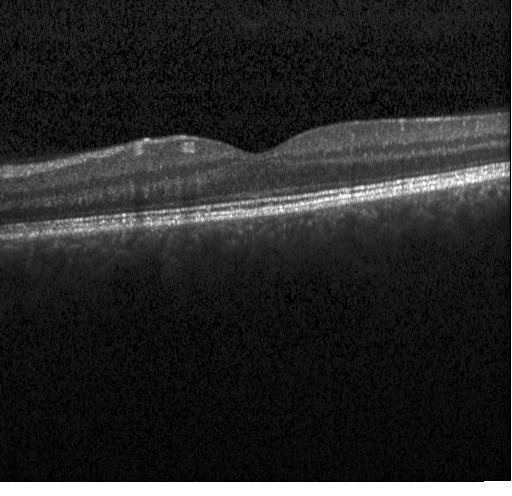 Retinal OCT cross-section. Impression: no choroidal neovascularization, diabetic macular edema, or drusen.